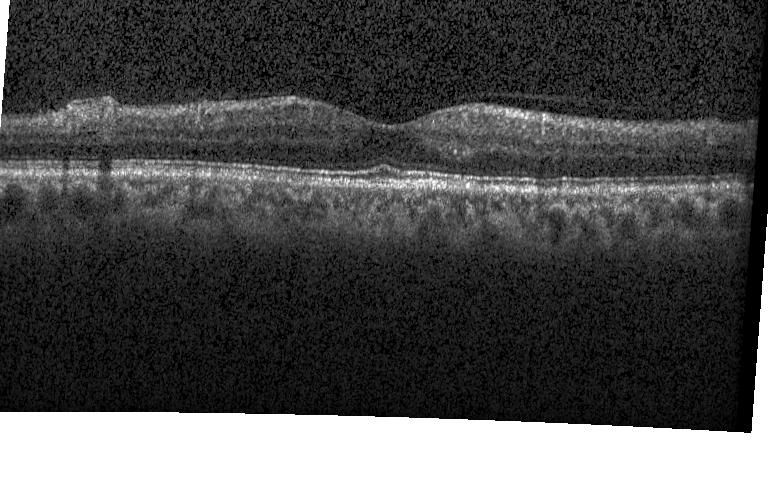
Impression: no evidence of CNV, DME, or drusen.